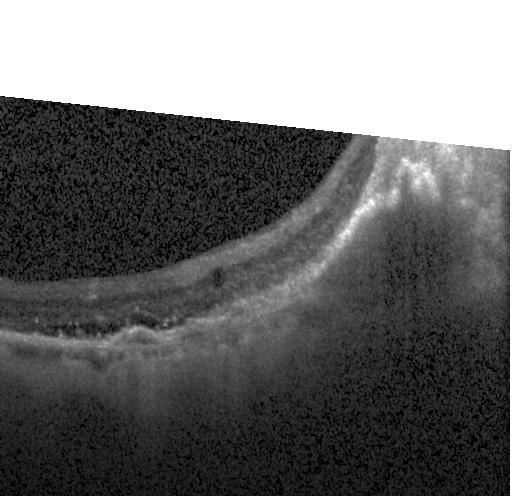
Optical coherence tomography scan; fovea-centered; instrument: Heidelberg Spectralis; SD-OCT. Diagnosis: choroidal neovascularization.